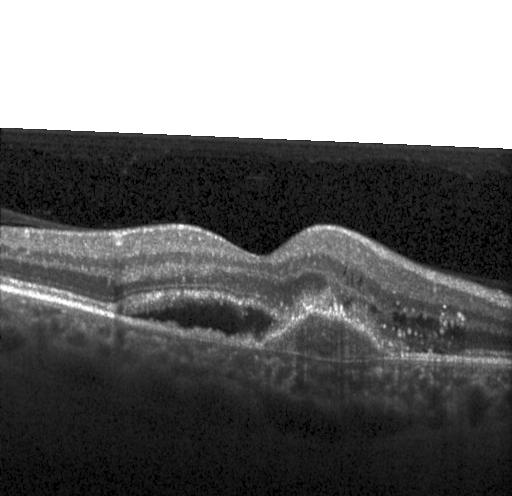 This B-scan demonstrates choroidal neovascularization (CNV).